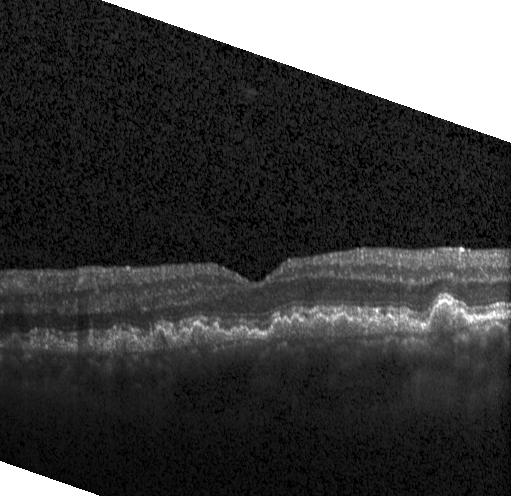
Macular OCT: a choroidal neovascular membrane.